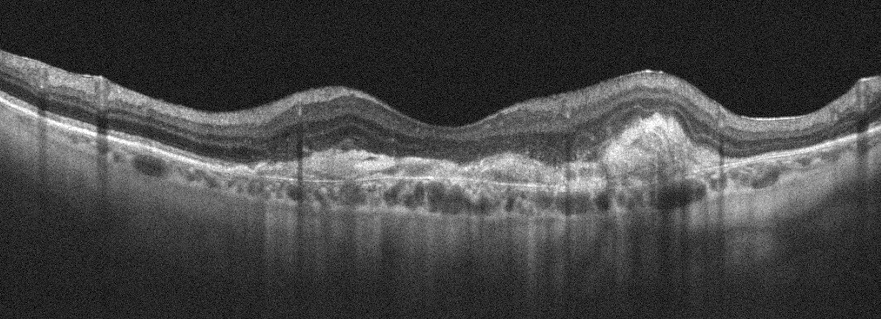
Retinal OCT B-scan, acquired on an Optovue Avanti RTVue XR, through the macula. Macular OCT: AMD.